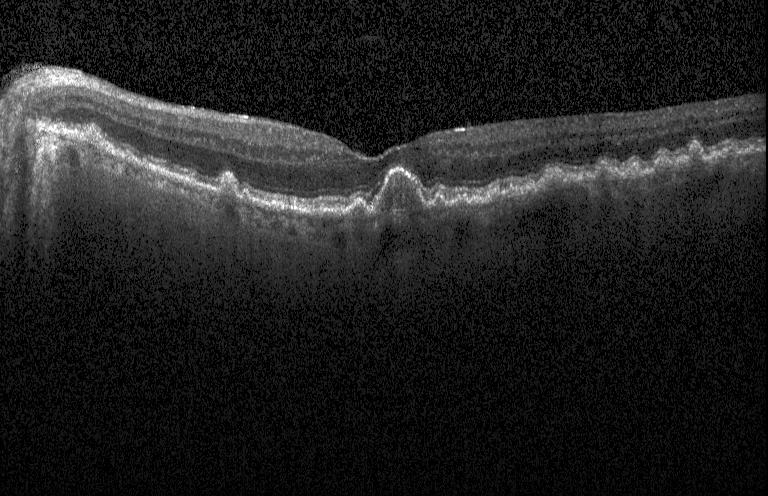 SD-OCT, OCT line scan — Assessment: multiple drusen.